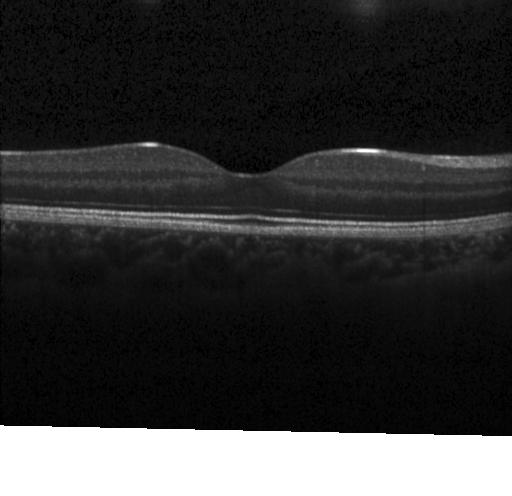

No evidence of CNV, DME, or drusen.